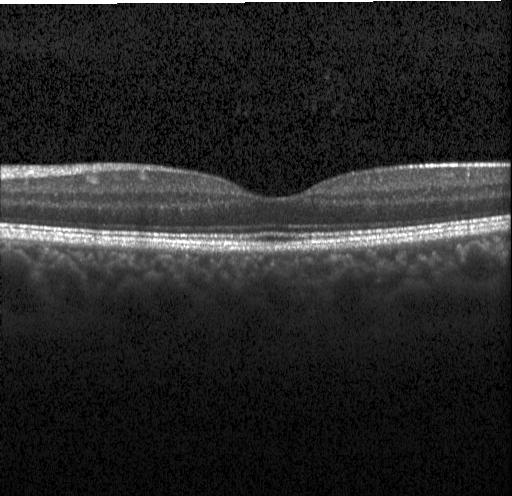 Dx: no CNV, DME, or drusen.